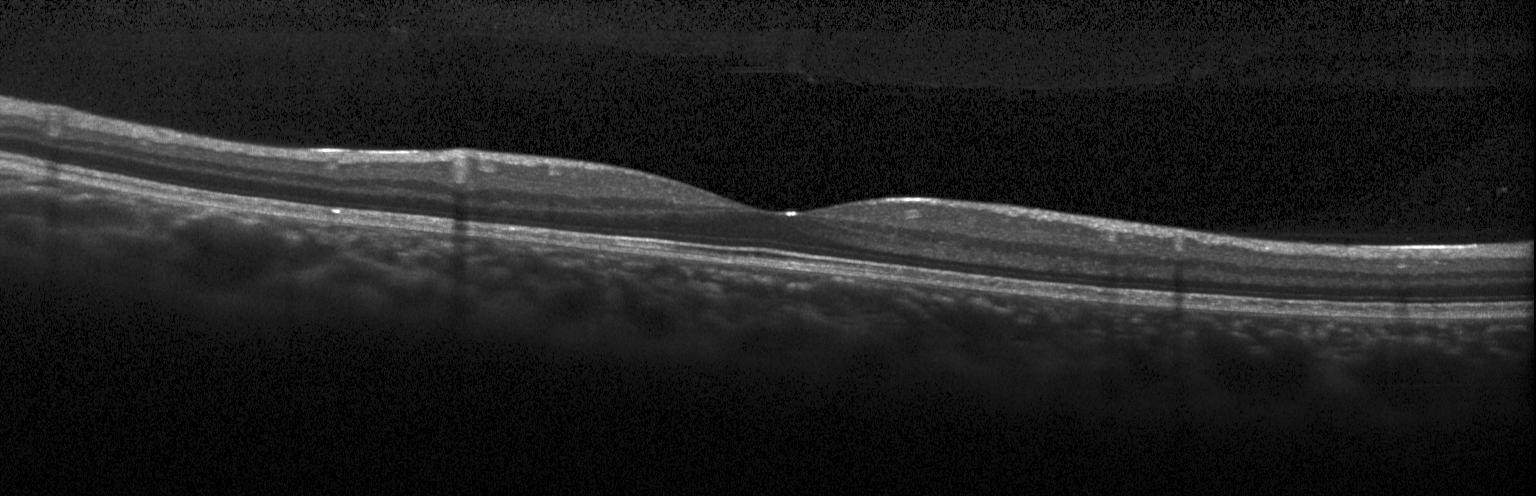 Retinal OCT cross-section showing no evidence of CNV, DME, or drusen.